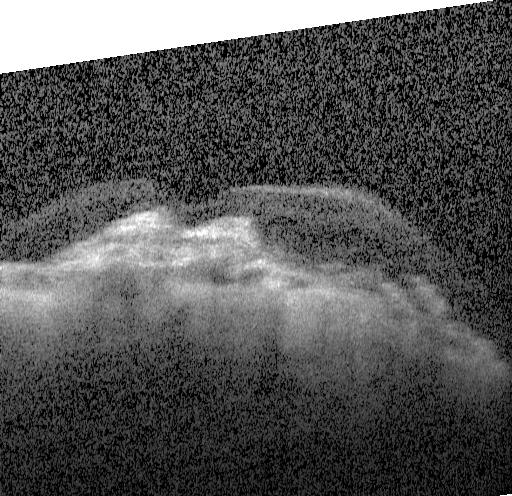 OCT B-scan.
The scan shows a choroidal neovascular membrane.